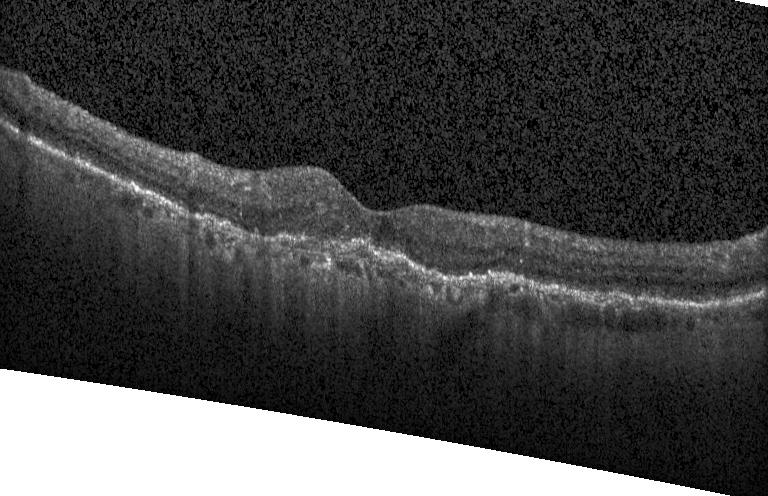
Macular OCT demonstrating a choroidal neovascular membrane.